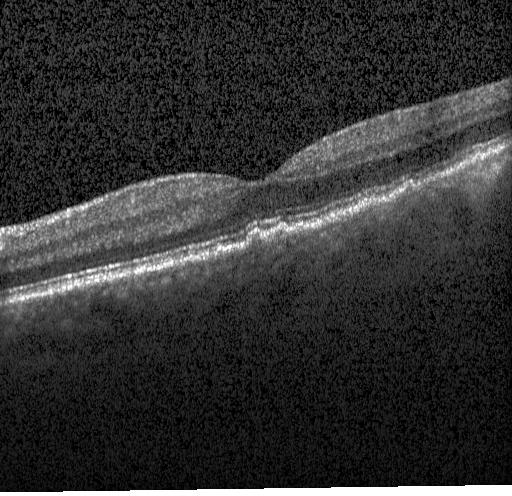

Drusen.